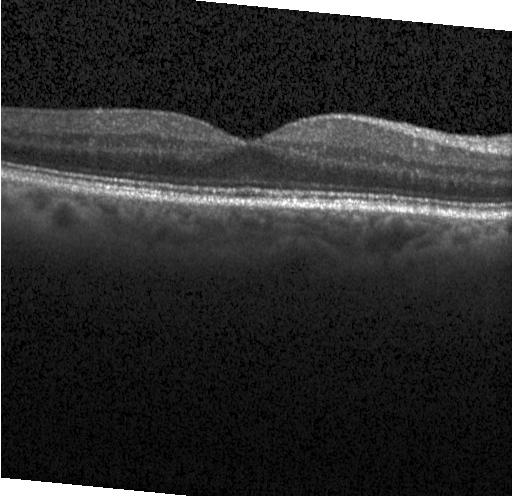
Centered on the fovea, optical coherence tomography B-scan, spectral-domain optical coherence tomography. Assessment: neither CNV, DME, nor drusen.